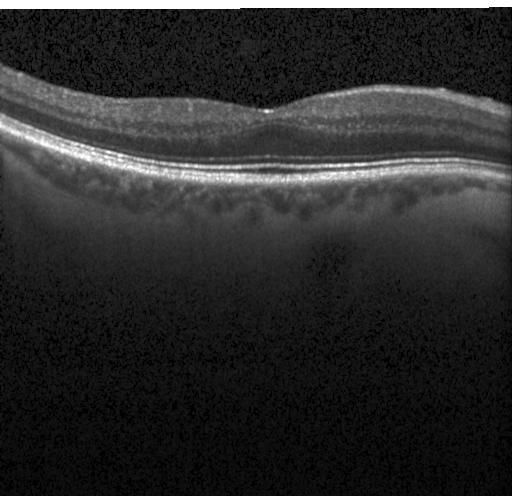 Impression: neither choroidal neovascularization, diabetic macular edema, nor drusen.